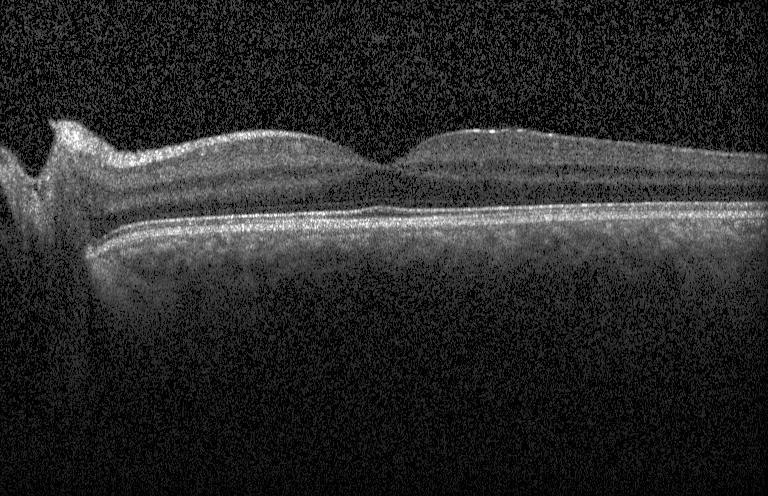
Instrument: Heidelberg Spectralis, fovea-centered, optical coherence tomography B-scan
Diagnosis: no evidence of choroidal neovascularization, diabetic macular edema, or drusen.